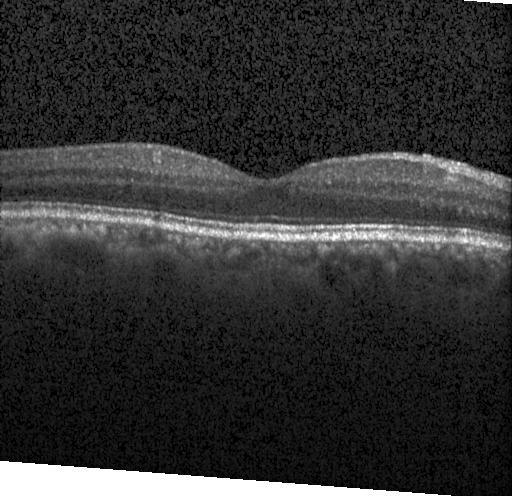

Optical coherence tomography scan, SD-OCT, macular scan. The scan shows no evidence of choroidal neovascularization, diabetic macular edema, or drusen.